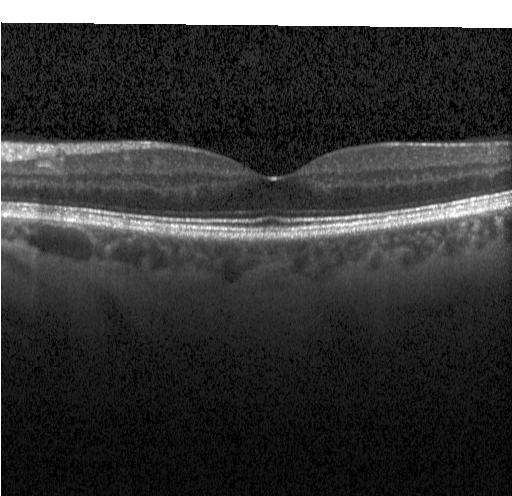

Fovea-centered, acquired on a Heidelberg Spectralis, OCT line scan, spectral-domain optical coherence tomography
The scan shows no evidence of choroidal neovascularization, diabetic macular edema, or drusen.